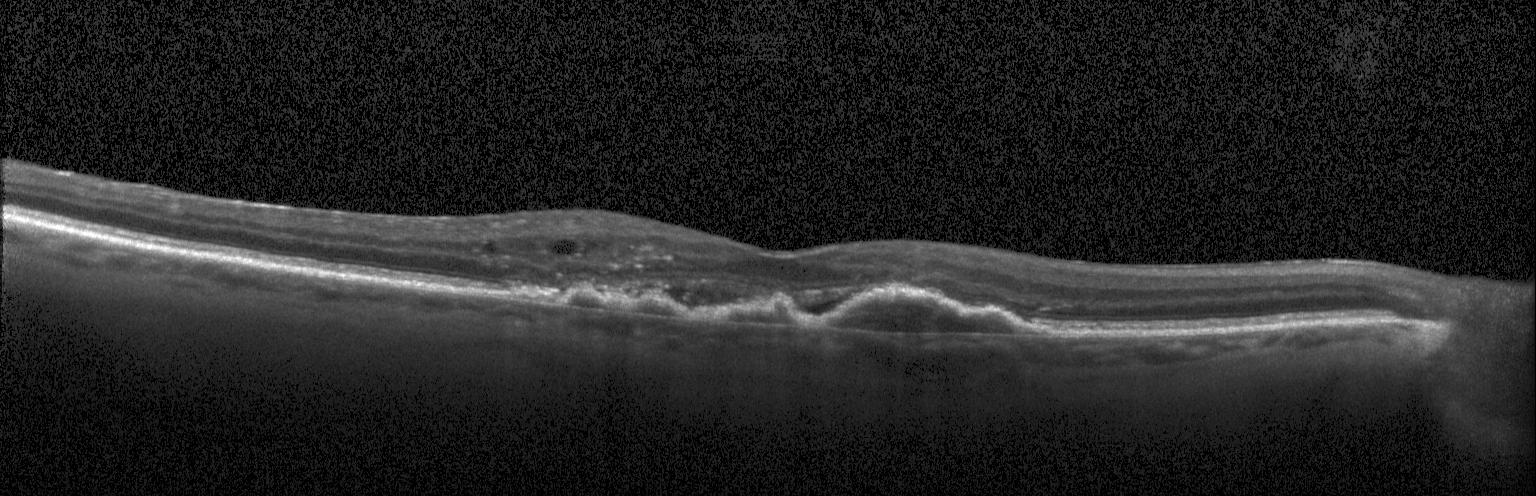 Horizontal scan through the fovea. Instrument: Heidelberg Spectralis. Optical coherence tomography scan — The scan shows a choroidal neovascular membrane.